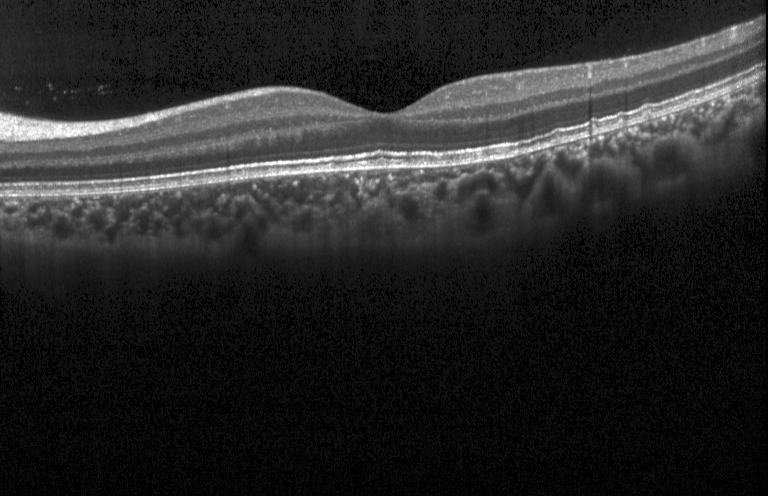 Macular scan; Heidelberg Spectralis OCT system; OCT B-scan. The scan shows no CNV, no DME, and no drusen.